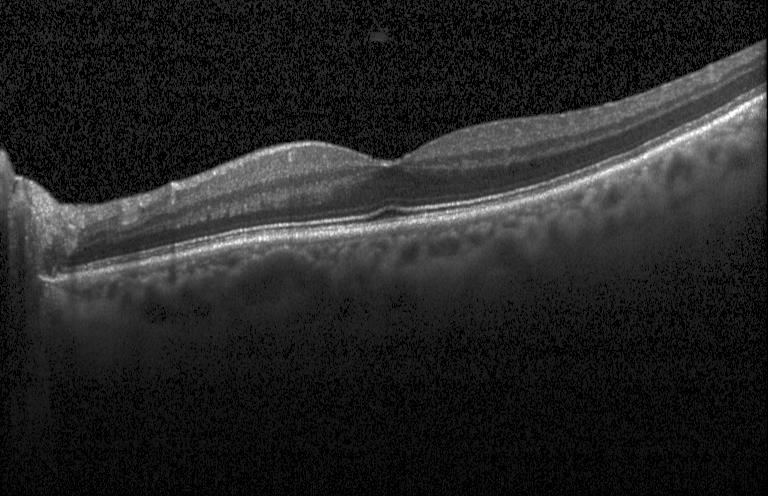 Spectral-domain optical coherence tomography · optical coherence tomography B-scan. Diagnosis: neither choroidal neovascularization, diabetic macular edema, nor drusen.